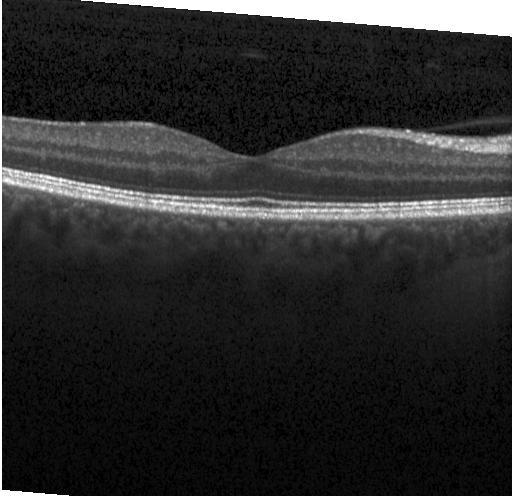 Acquired on a Heidelberg Spectralis; retinal OCT B-scan; horizontal scan through the fovea
Dx: no choroidal neovascularization, no diabetic macular edema, and no drusen.